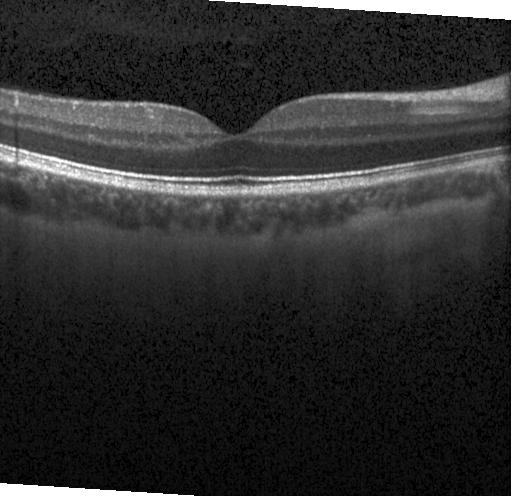
OCT B-scan — Diagnosis: neither CNV, DME, nor drusen.